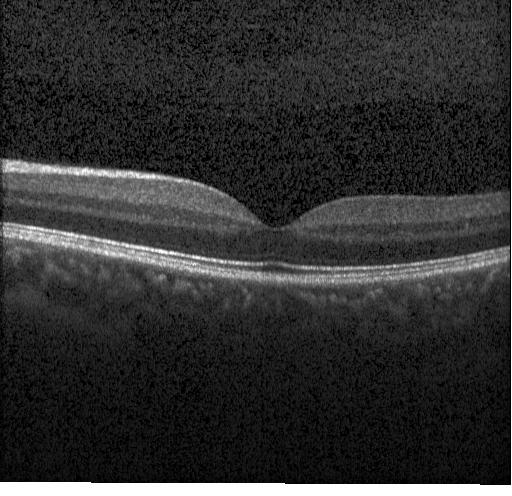
Diagnosis: no choroidal neovascularization, no diabetic macular edema, and no drusen.